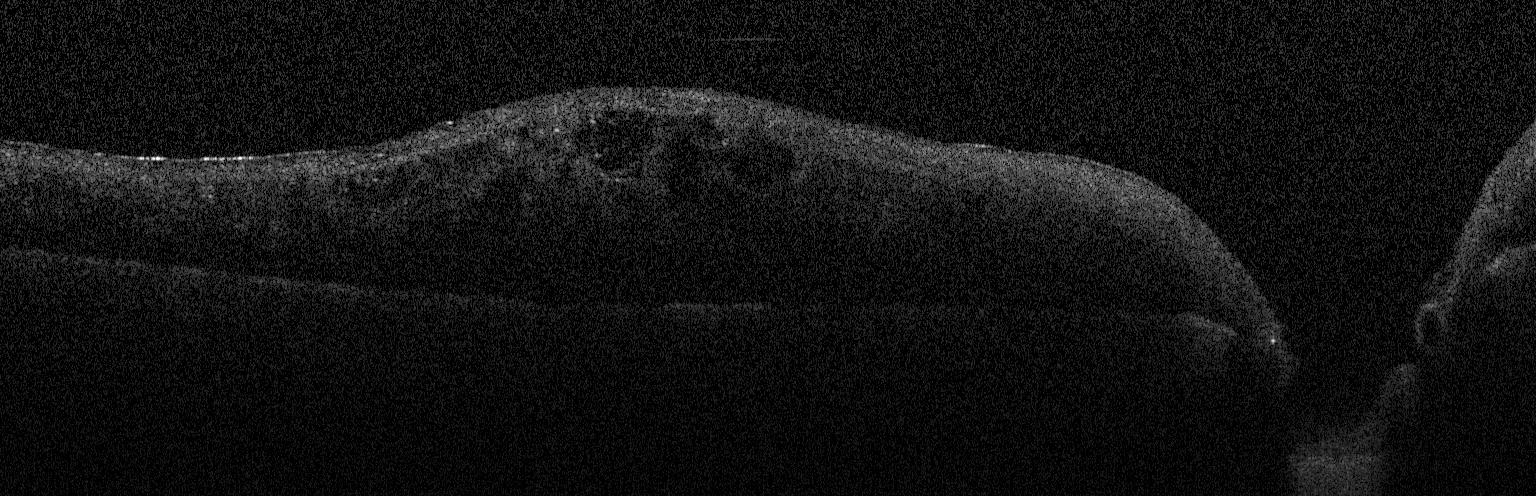

Centered on the fovea, optical coherence tomography scan, acquired on a Heidelberg Spectralis.
The scan shows DME.